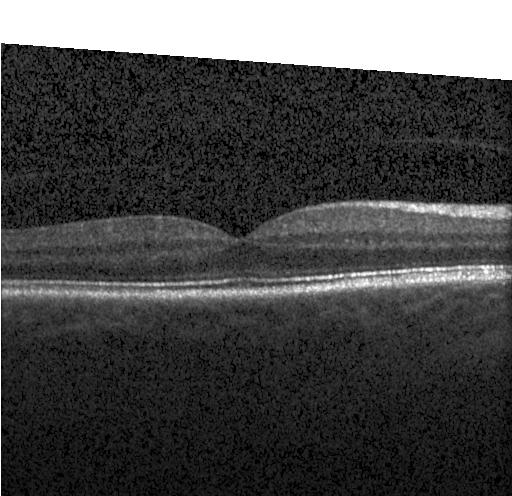 Optical coherence tomography B-scan. Acquired on a Heidelberg Spectralis. Spectral-domain OCT. Through the macula — This B-scan demonstrates no CNV, DME, or drusen.